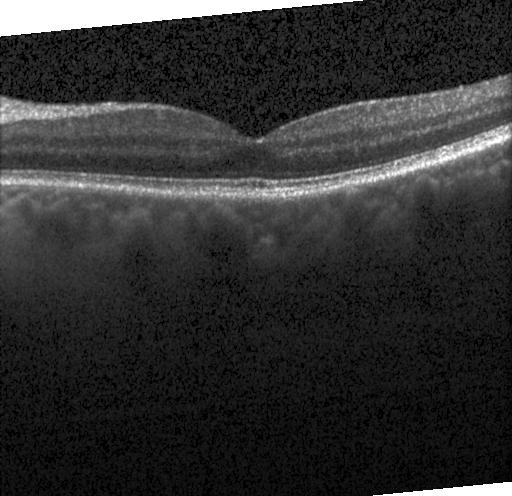
Acquired on a Heidelberg Spectralis; retinal OCT B-scan. Diagnosis: neither choroidal neovascularization, diabetic macular edema, nor drusen.